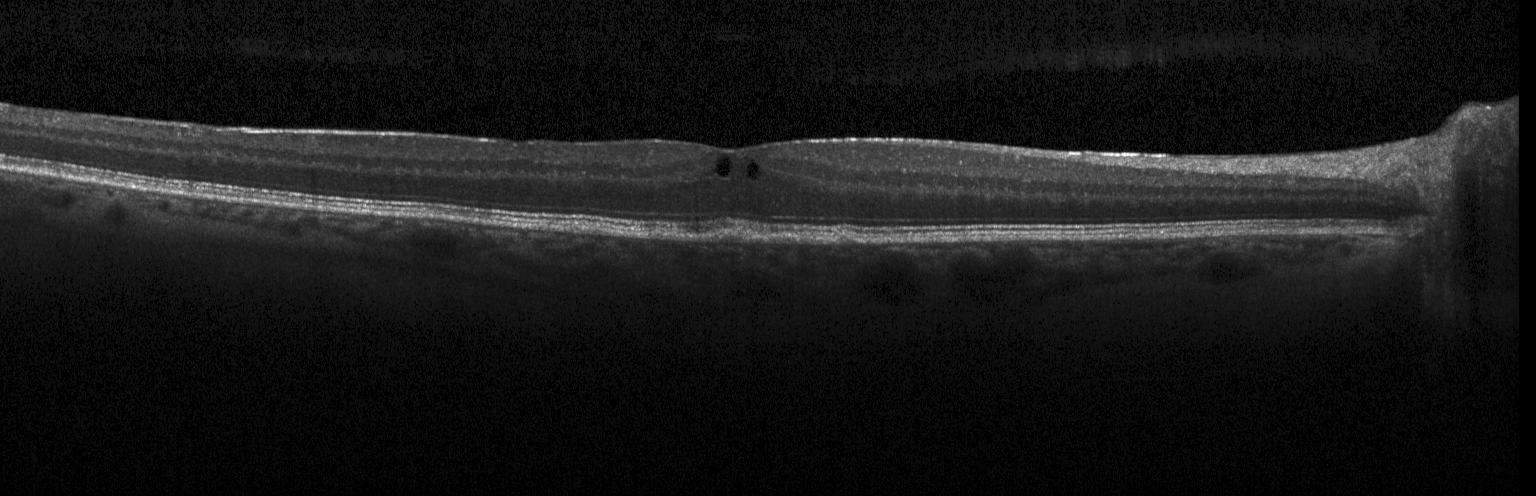
Optical coherence tomography scan
Assessment: diabetic macular edema (DME).